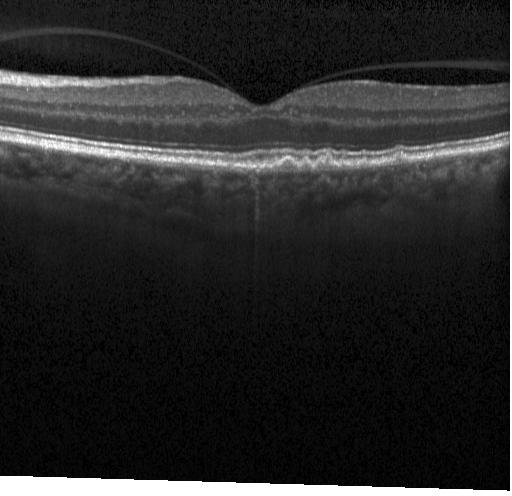
Retinal OCT cross-section; acquired on a Heidelberg Spectralis — Impression: sub-RPE drusenoid deposits.